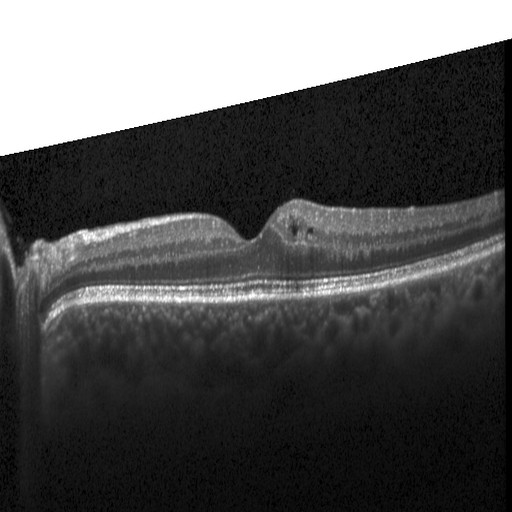

Assessment: diabetic macular edema.